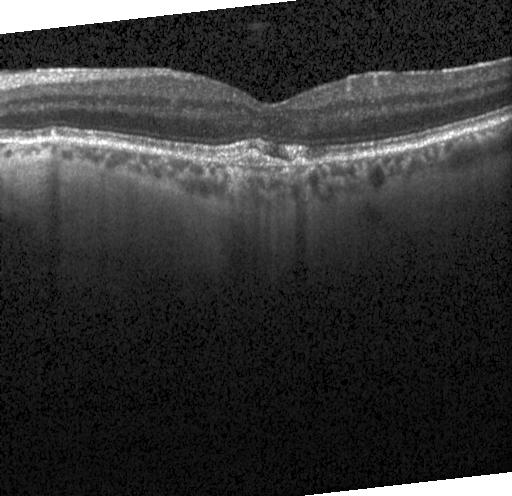
Spectral-domain OCT B-scan: a choroidal neovascular membrane.